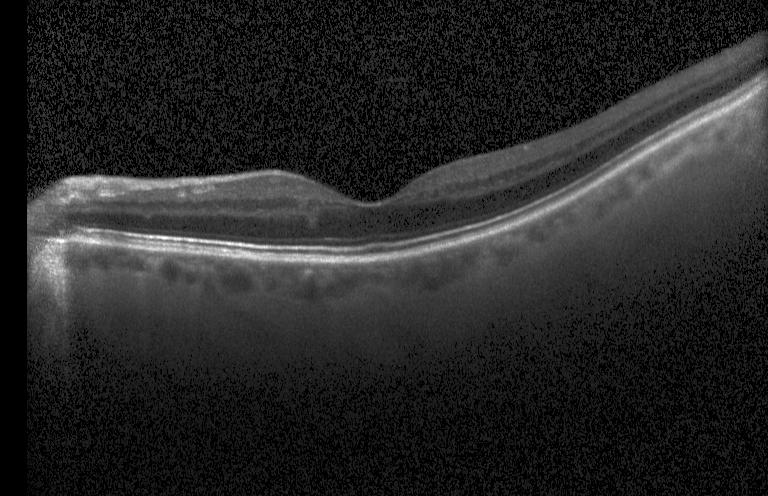
Spectral-domain OCT. Fovea-centered. Acquired on a Heidelberg Spectralis. OCT B-scan. Impression: no evidence of choroidal neovascularization, diabetic macular edema, or drusen.